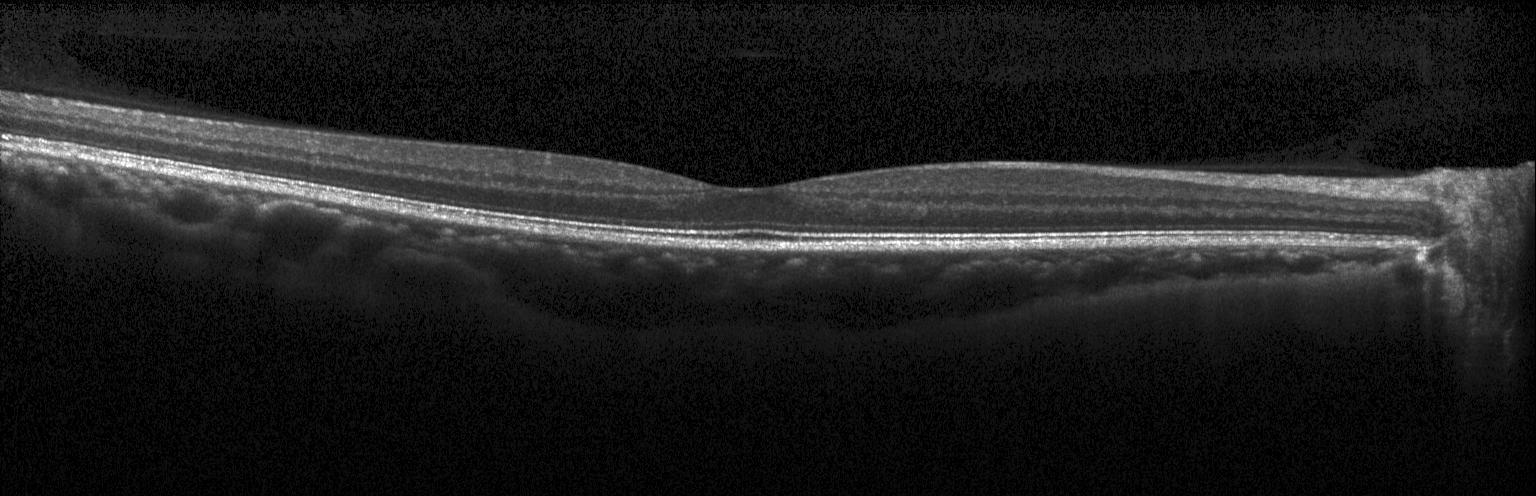 Centered on the fovea · spectral-domain optical coherence tomography · optical coherence tomography scan.
Finding: no CNV, DME, or drusen.